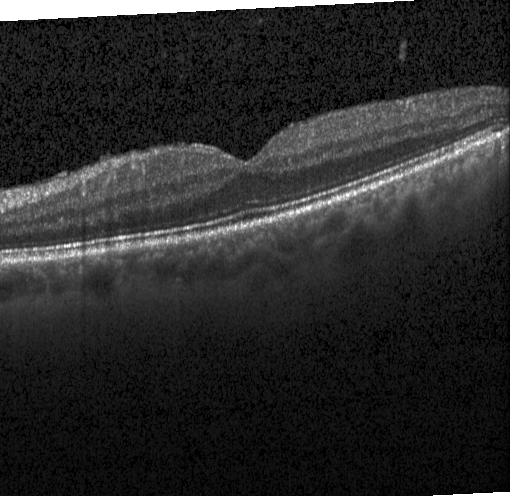 Diagnosis: neither choroidal neovascularization, diabetic macular edema, nor drusen.